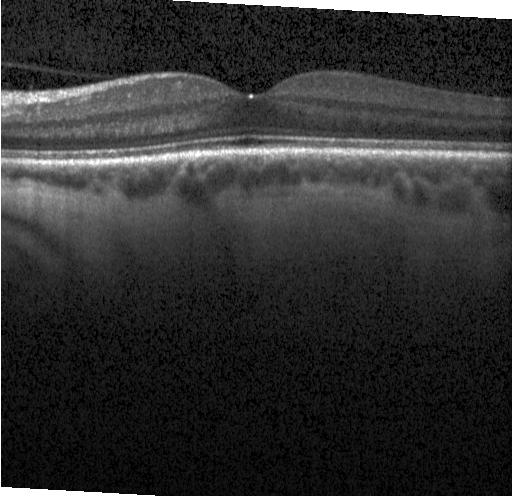
No choroidal neovascularization, diabetic macular edema, or drusen.